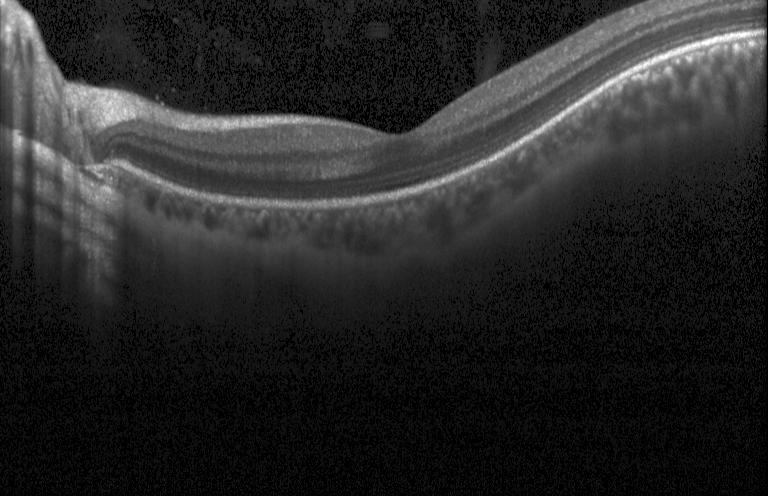 Finding: no choroidal neovascularization, diabetic macular edema, or drusen.